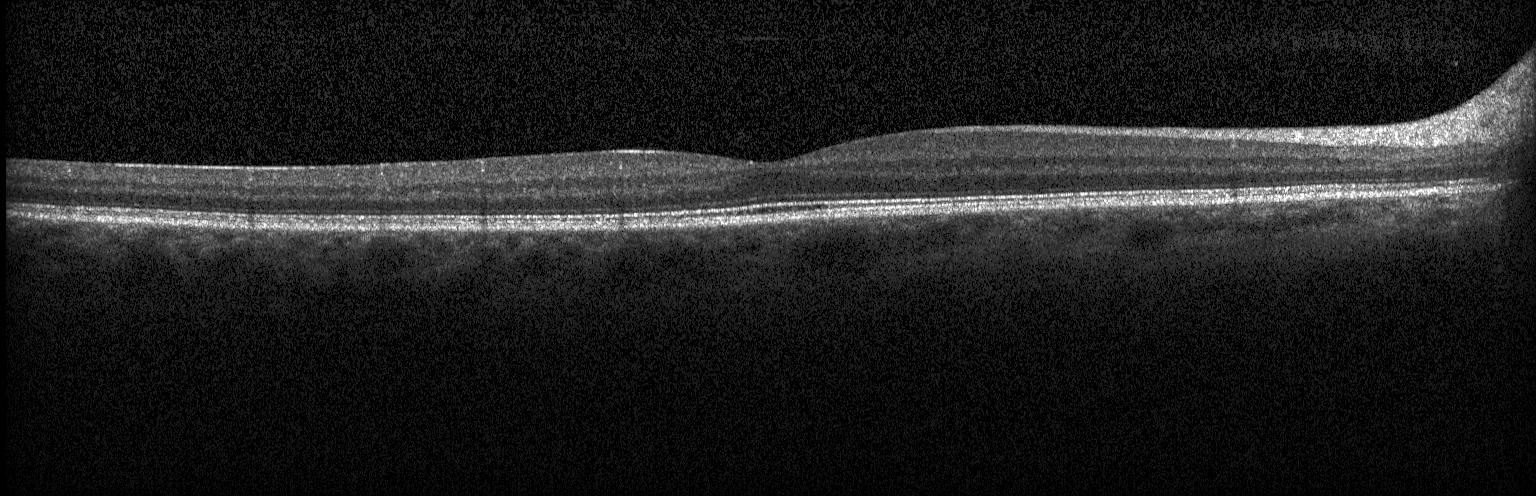

Centered on the fovea; optical coherence tomography B-scan; spectral-domain OCT. The scan shows no evidence of choroidal neovascularization, diabetic macular edema, or drusen.